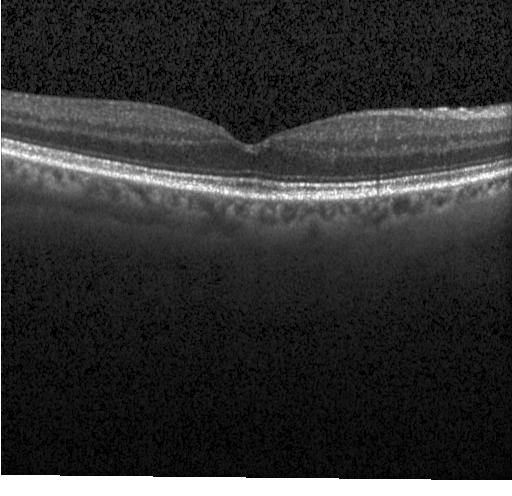

OCT line scan.
Assessment: no choroidal neovascularization, diabetic macular edema, or drusen.